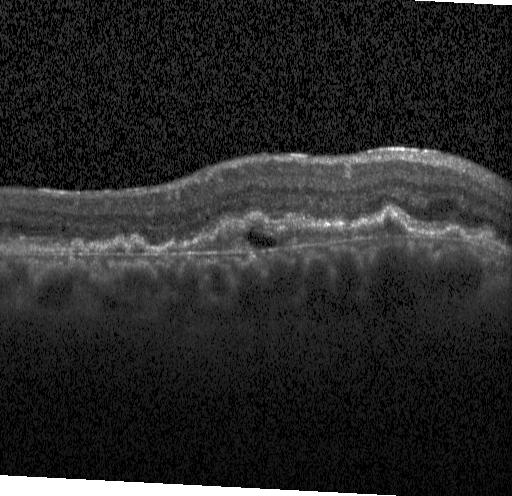 OCT finding: choroidal neovascularization (CNV).